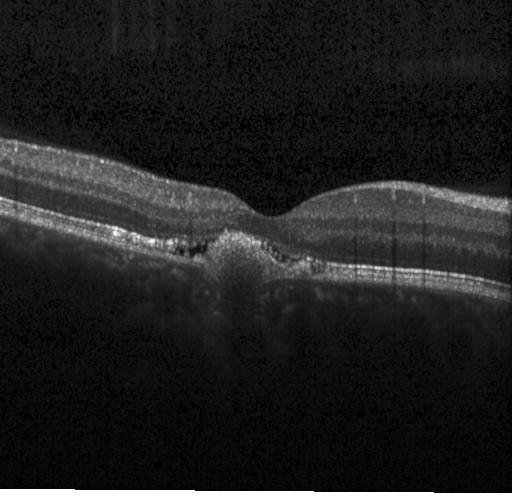 Optical coherence tomography scan · spectral-domain OCT · Heidelberg Spectralis · macular scan. The scan shows a choroidal neovascular membrane.